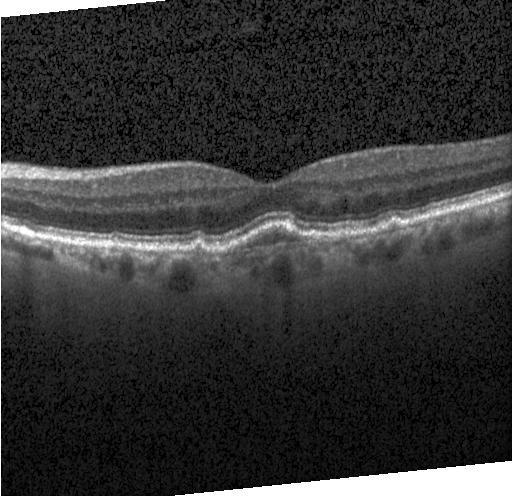
Choroidal neovascularization (CNV).